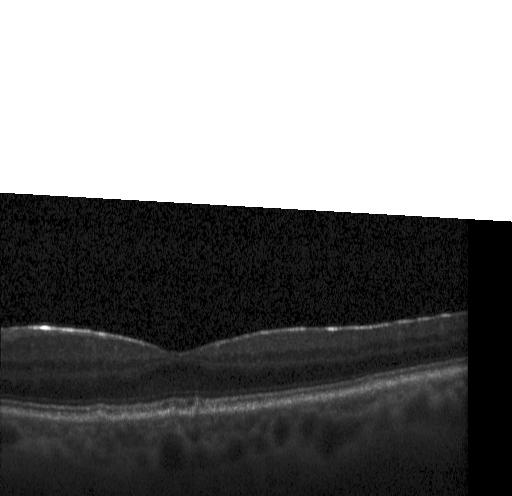
OCT scan showing sub-RPE drusenoid deposits.